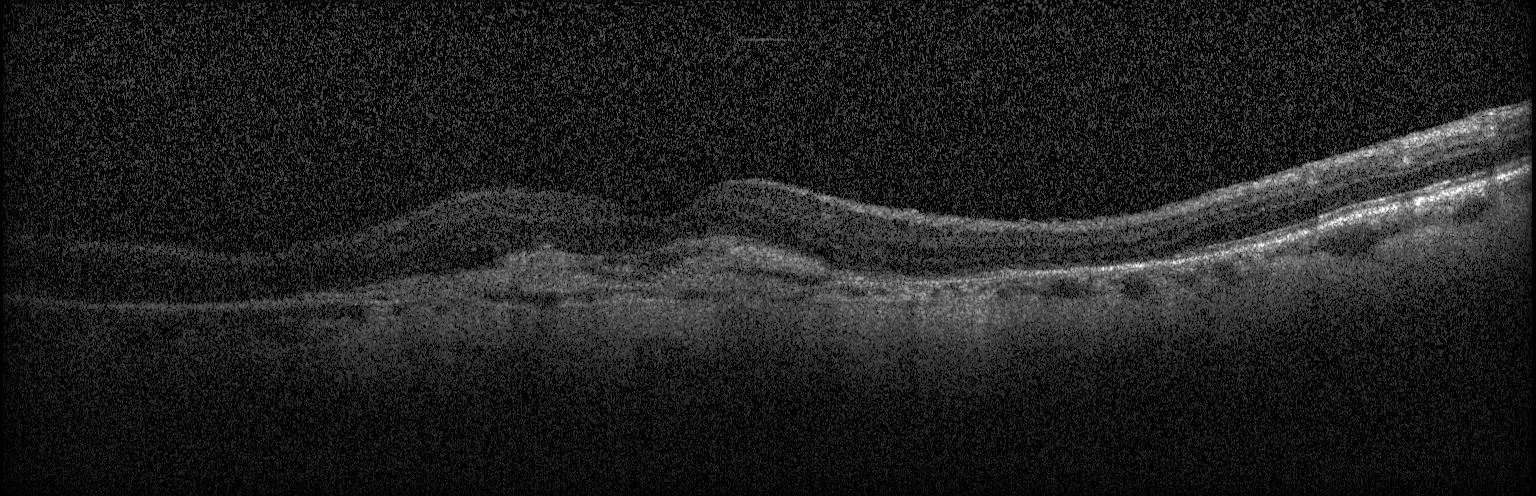

Heidelberg Spectralis OCT system. Fovea-centered. Retinal OCT B-scan. SD-OCT
Diagnosis: CNV.